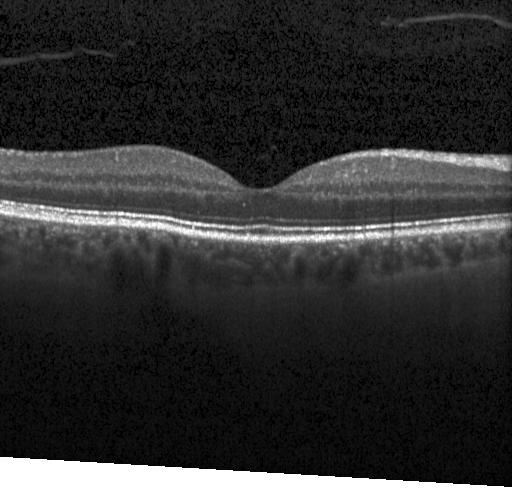 Impression: no CNV, no DME, and no drusen.